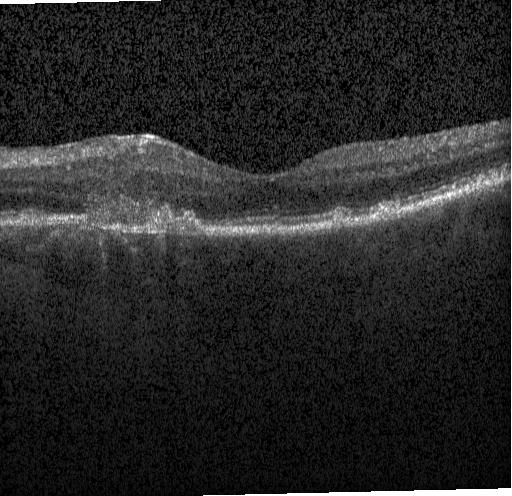
Finding: choroidal neovascularization.